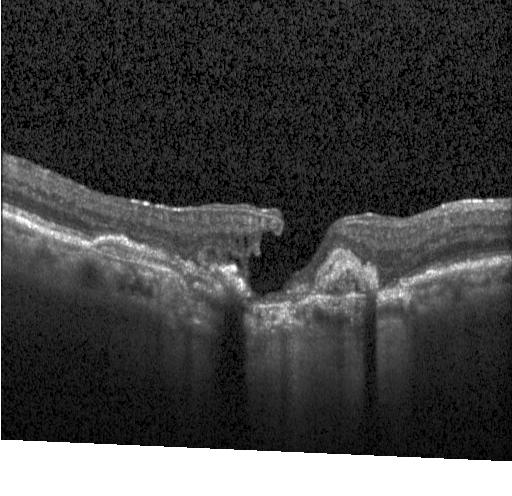
Macular OCT: a choroidal neovascular membrane.